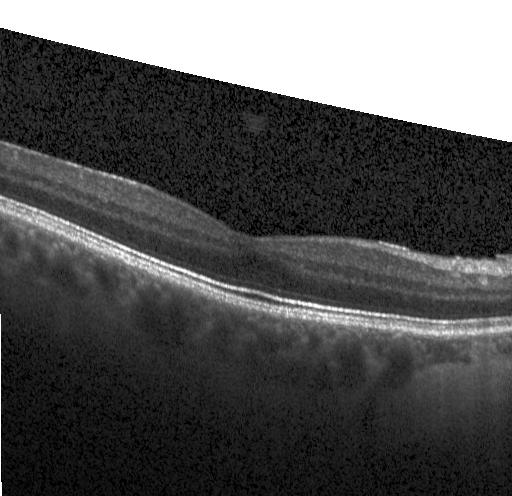

Assessment: no evidence of CNV, DME, or drusen.